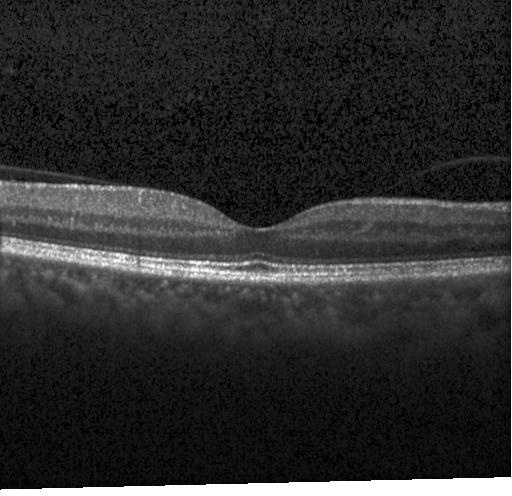 Retinal OCT cross-section. Heidelberg Spectralis. Horizontal scan through the fovea
Assessment: neither CNV, DME, nor drusen.